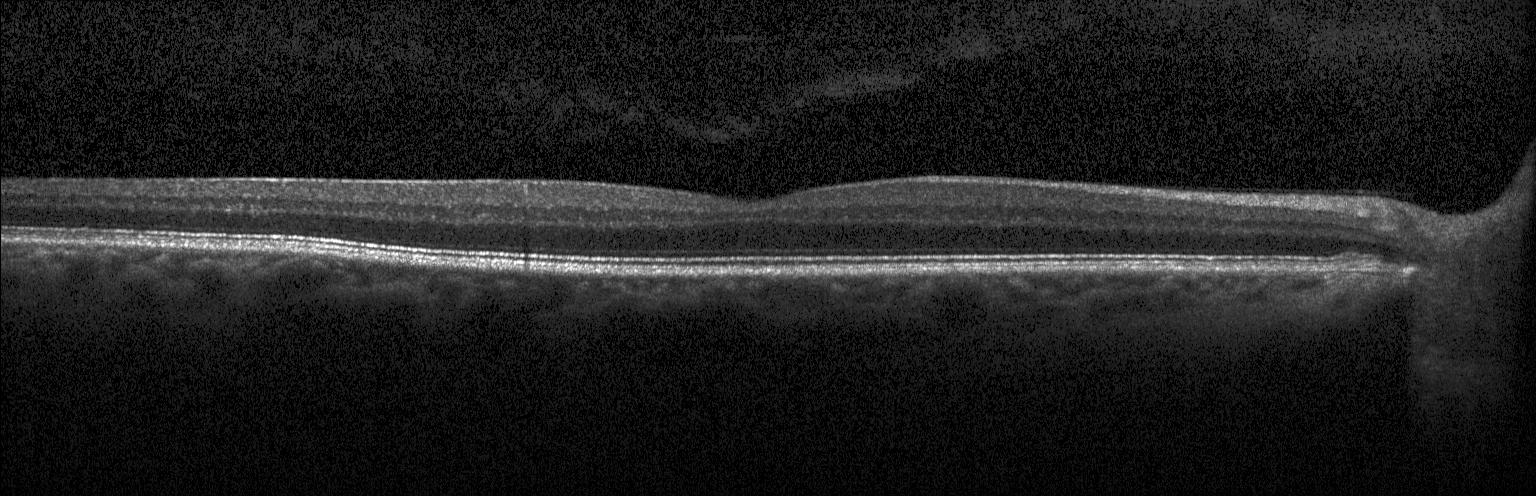
Fovea-centered · retinal OCT B-scan · Heidelberg Spectralis OCT system · spectral-domain optical coherence tomography.
Diagnosis: neither choroidal neovascularization, diabetic macular edema, nor drusen.